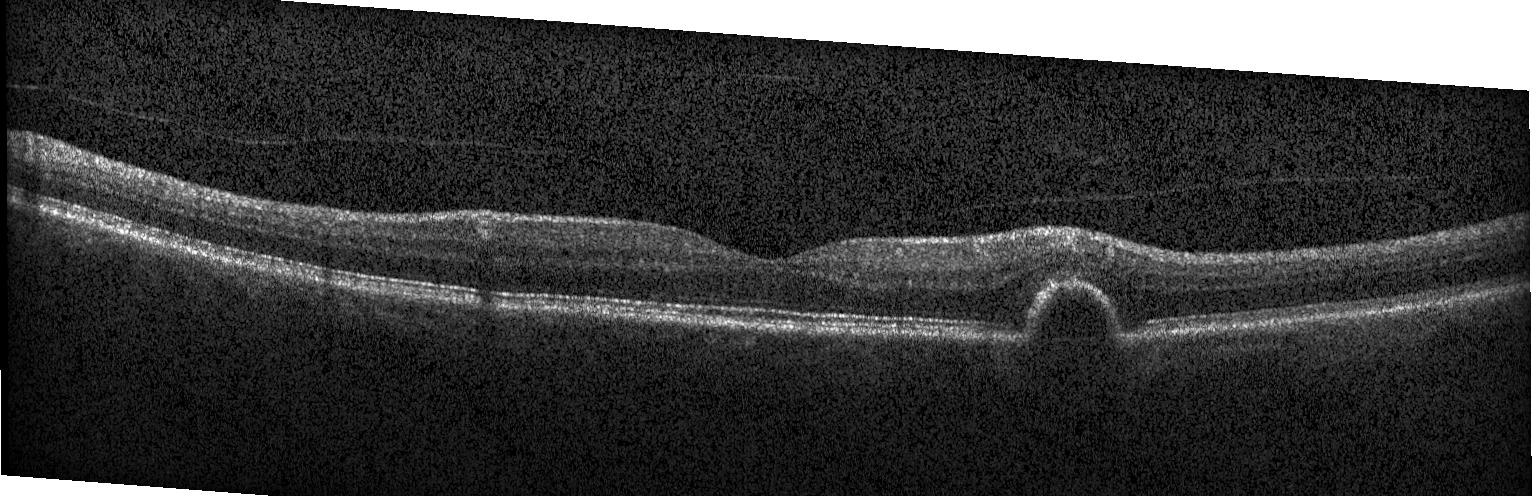
Retinal OCT cross-section.
Diagnosis: choroidal neovascularization (CNV).